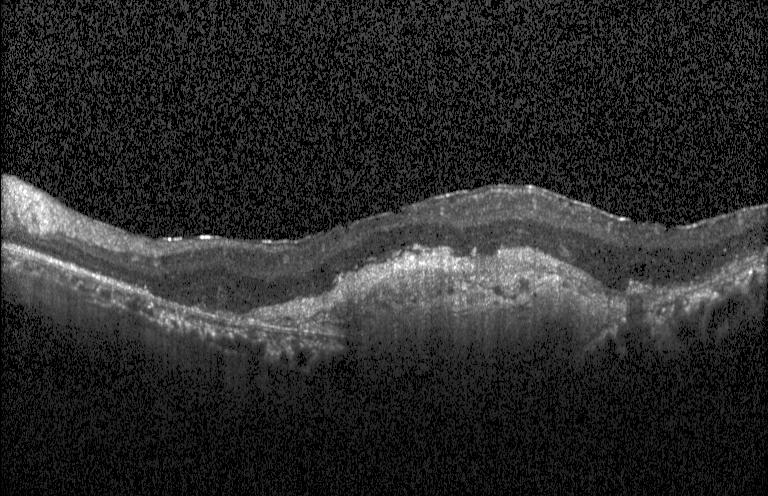

SD-OCT · macular scan · Heidelberg Spectralis · optical coherence tomography scan — Finding: CNV.